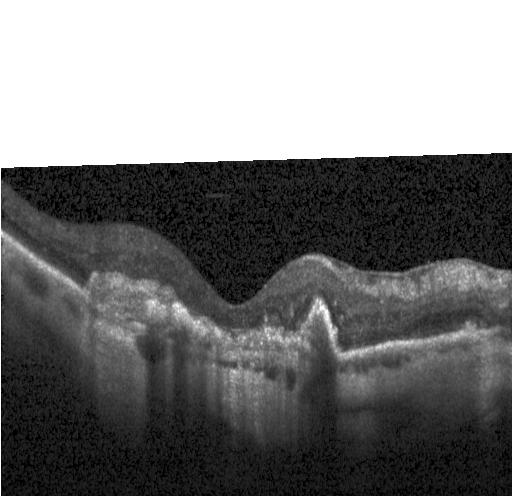
Spectral-domain optical coherence tomography, acquired on a Heidelberg Spectralis, OCT line scan. Finding: a choroidal neovascular membrane.